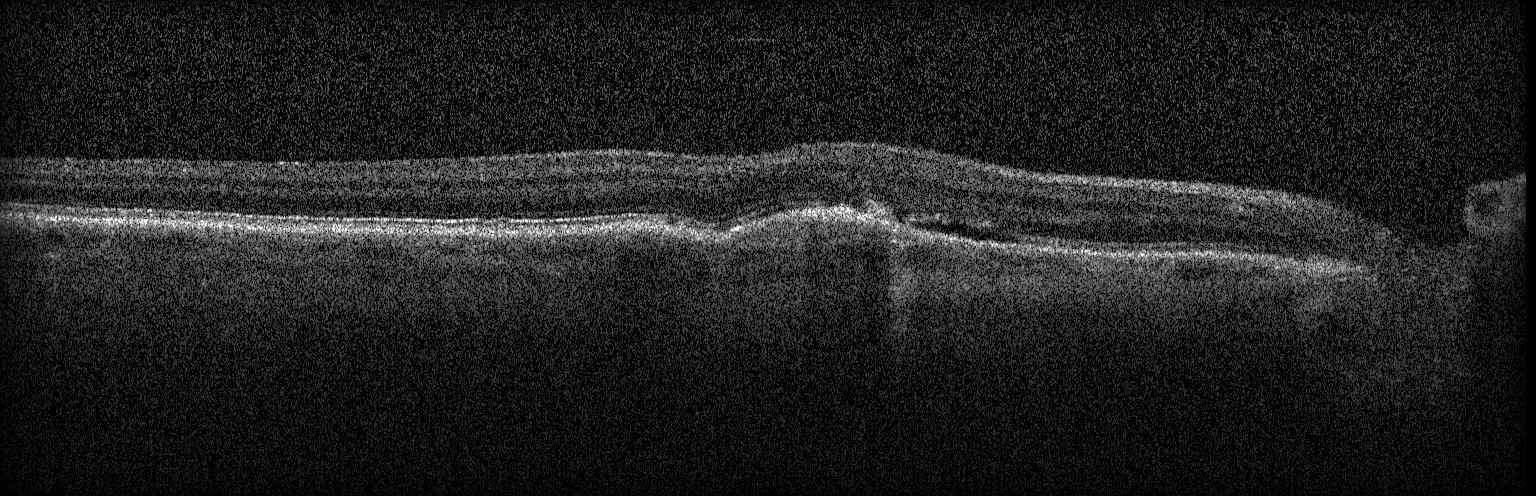 Optical coherence tomography scan, acquired on a Heidelberg Spectralis, centered on the fovea. Impression: a choroidal neovascular membrane.